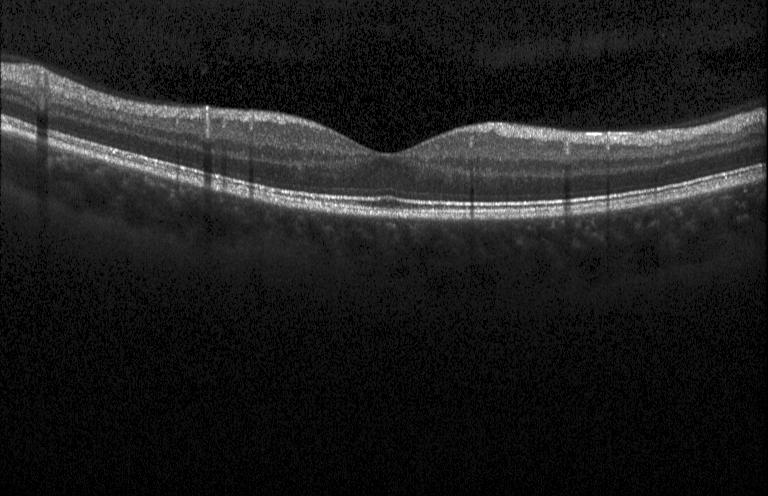

OCT finding: neither choroidal neovascularization, diabetic macular edema, nor drusen.